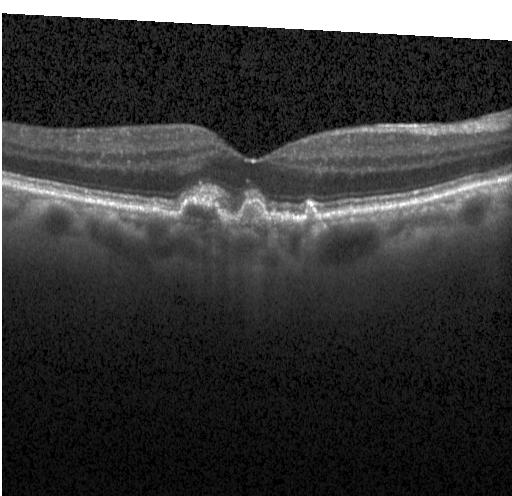
Spectral-domain OCT B-scan: choroidal neovascularization.